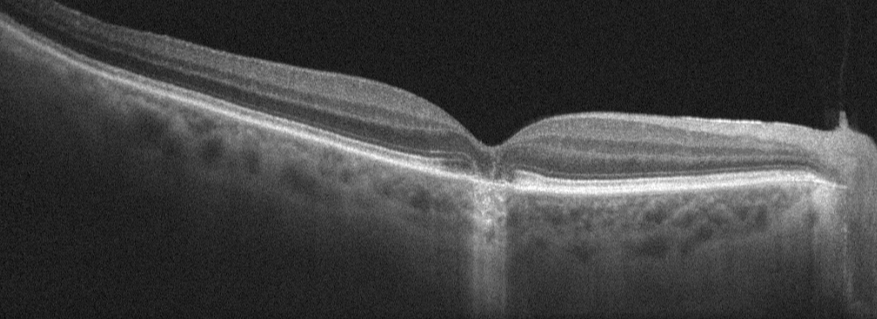

Retinal OCT cross-section.
Diagnosis: age-related macular degeneration.